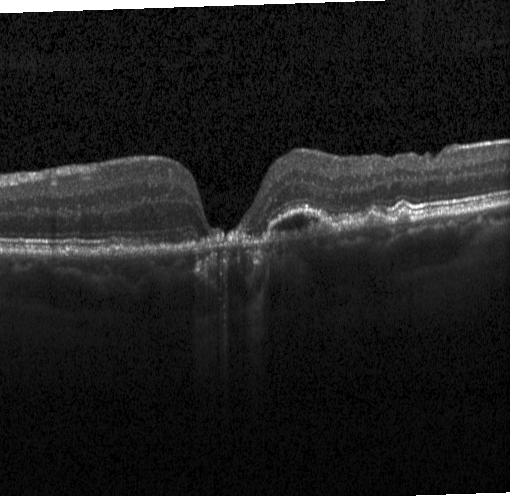
Horizontal scan through the fovea · retinal OCT cross-section · Heidelberg Spectralis
OCT finding: a choroidal neovascular membrane.